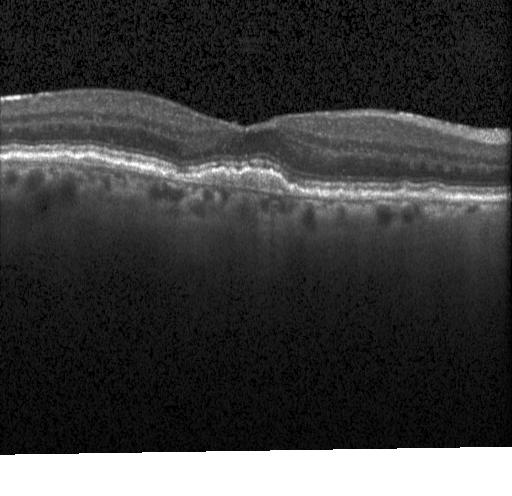

Optical coherence tomography B-scan.
Choroidal neovascularization (CNV).